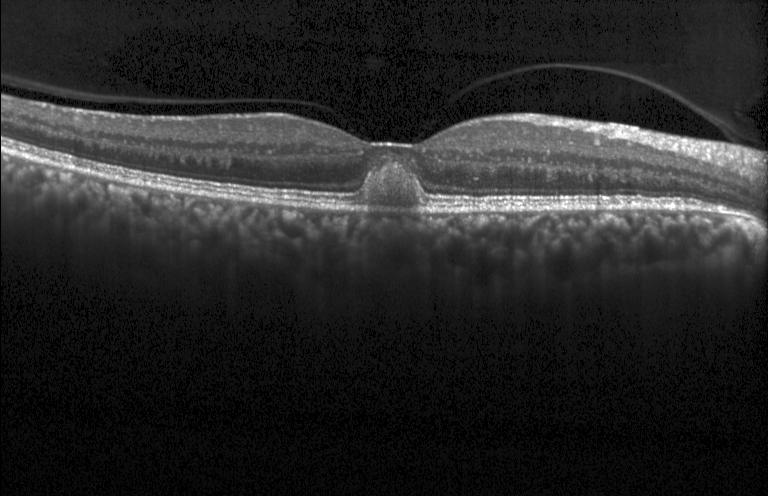 Heidelberg Spectralis; optical coherence tomography B-scan
Diagnosis: a choroidal neovascular membrane.